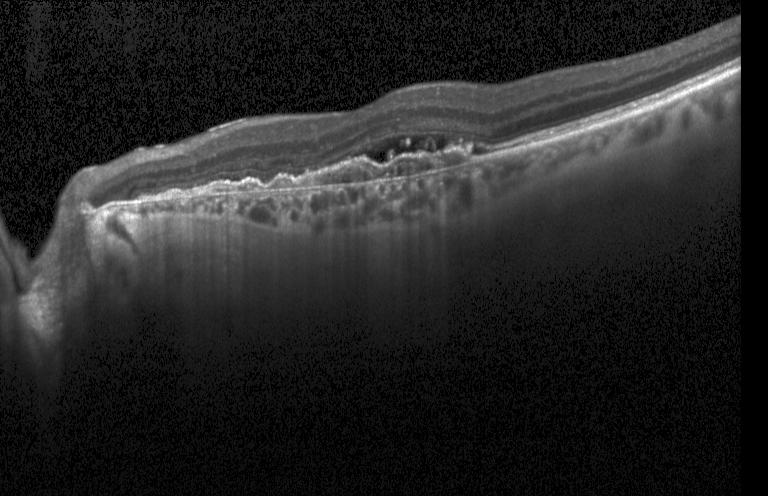

Macular OCT: choroidal neovascularization.